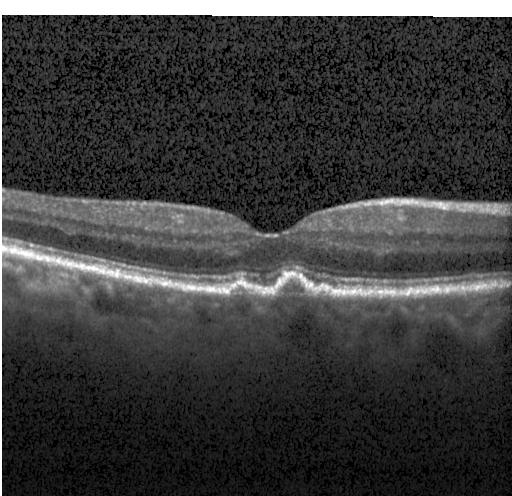

The scan shows sub-RPE drusenoid deposits.